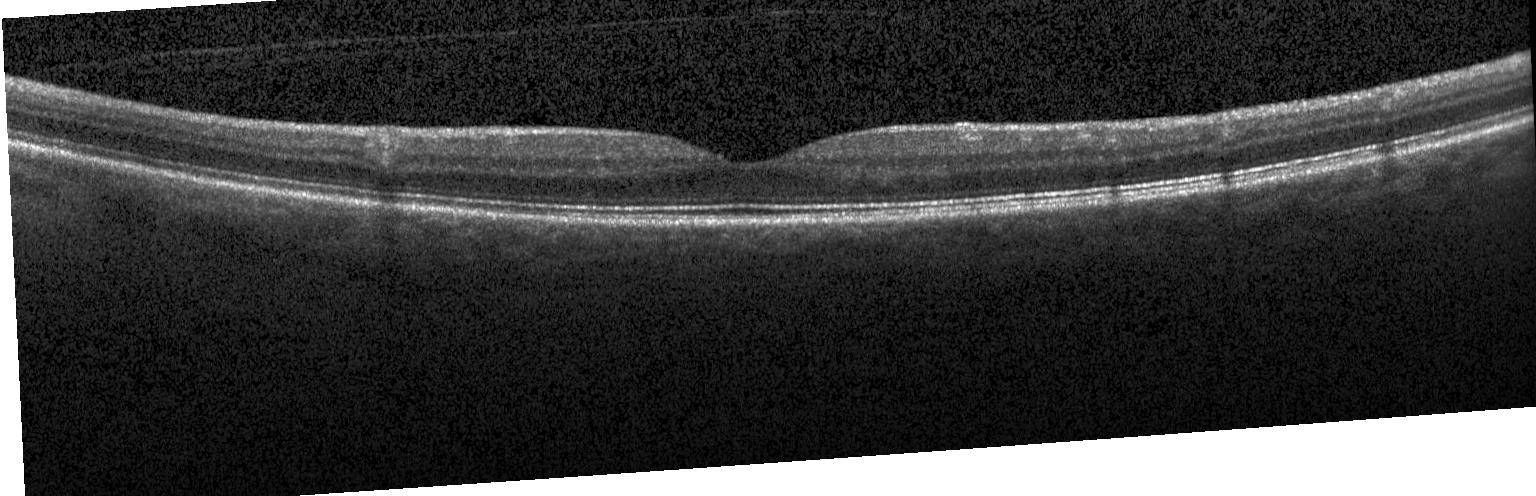

The scan shows neither choroidal neovascularization, diabetic macular edema, nor drusen.